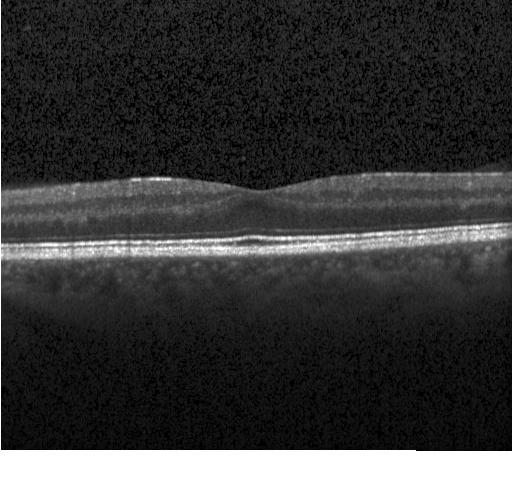 Optical coherence tomography B-scan. Diagnosis: no evidence of choroidal neovascularization, diabetic macular edema, or drusen.